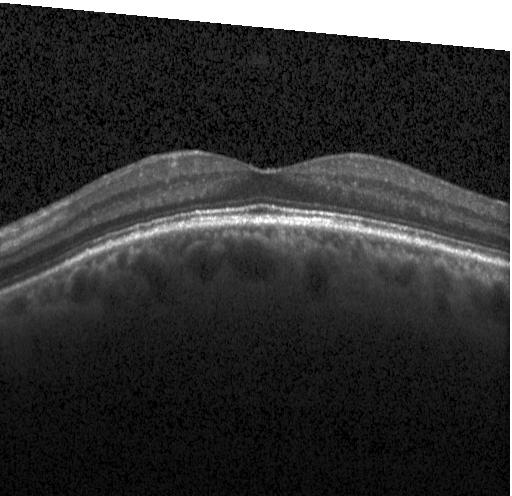 Heidelberg Spectralis OCT system; retinal OCT B-scan; macular scan; SD-OCT.
Macular OCT: no choroidal neovascularization, no diabetic macular edema, and no drusen.